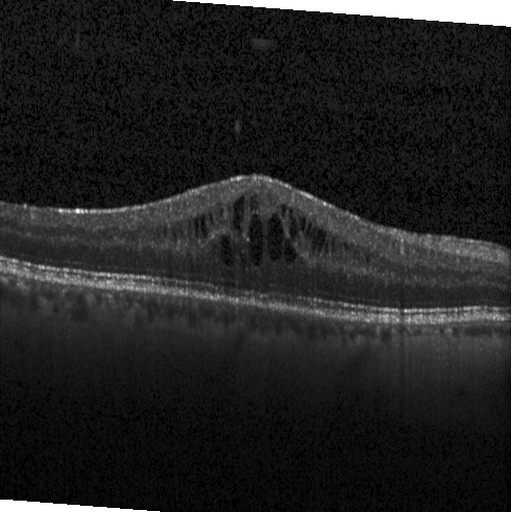

Finding: diabetic macular edema (DME).